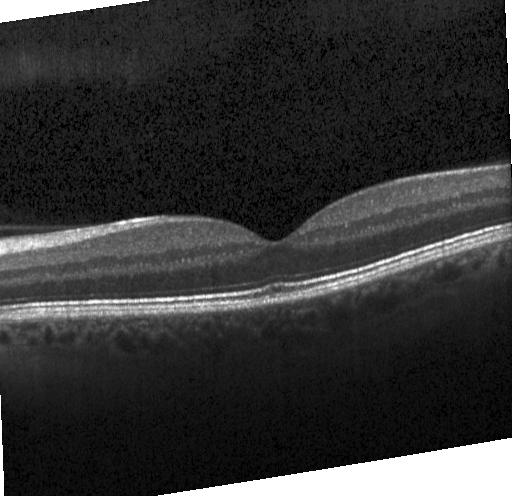

OCT finding: no CNV, DME, or drusen.